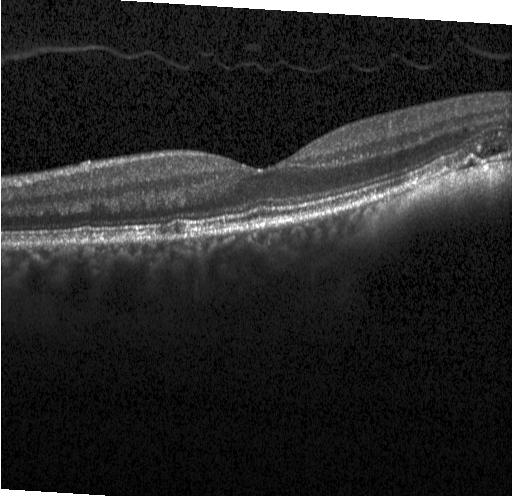 Finding: a choroidal neovascular membrane.